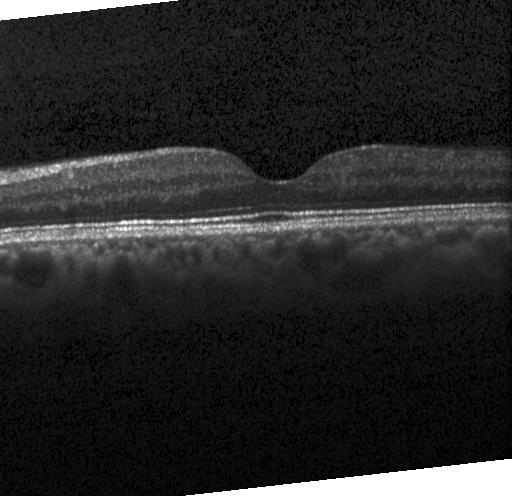

Spectral-domain optical coherence tomography · acquired on a Heidelberg Spectralis · horizontal scan through the fovea · OCT B-scan
This B-scan demonstrates no evidence of choroidal neovascularization, diabetic macular edema, or drusen.